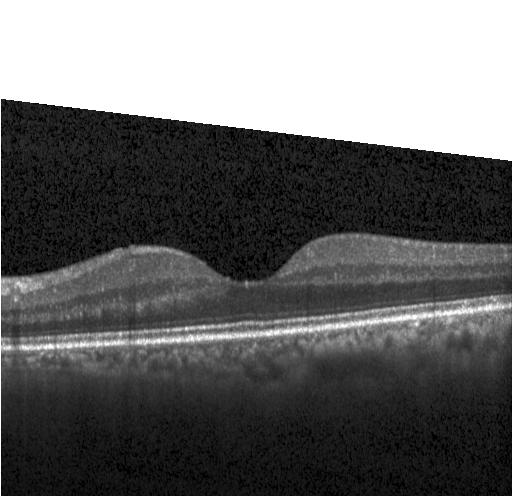

Acquired on a Heidelberg Spectralis, OCT line scan, macular scan.
Finding: no CNV, no DME, and no drusen.